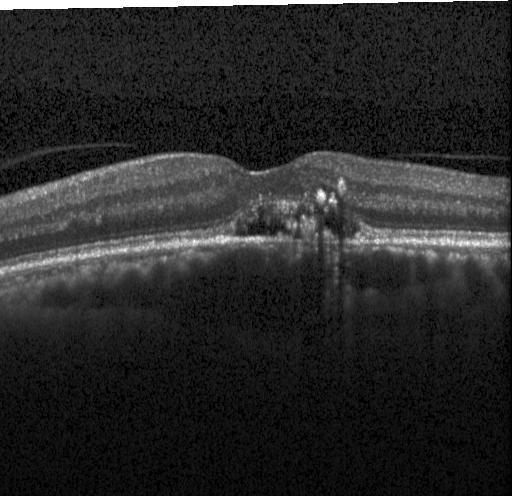
The scan shows choroidal neovascularization (CNV).